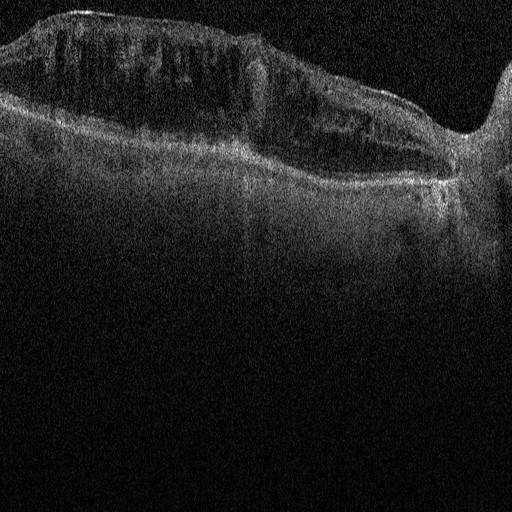

OCT line scan. Diabetic macular edema (DME).